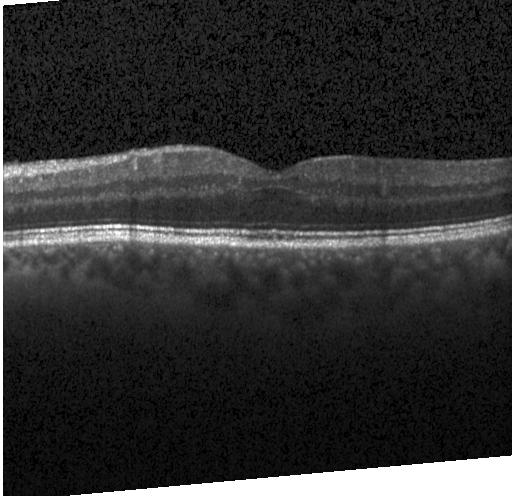
Retinal OCT cross-section showing neither choroidal neovascularization, diabetic macular edema, nor drusen.